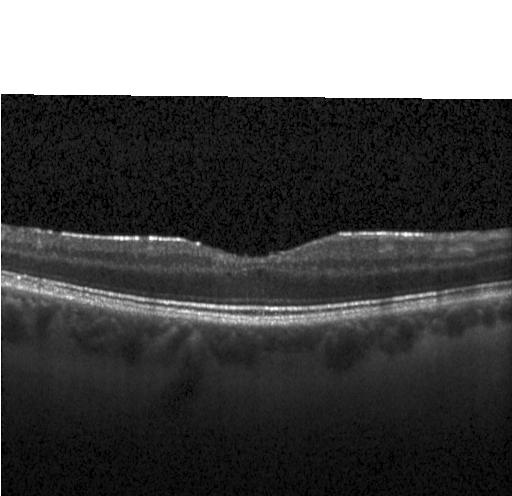 Instrument: Heidelberg Spectralis, spectral-domain optical coherence tomography, OCT B-scan, macular scan — Macular OCT: no CNV, DME, or drusen.